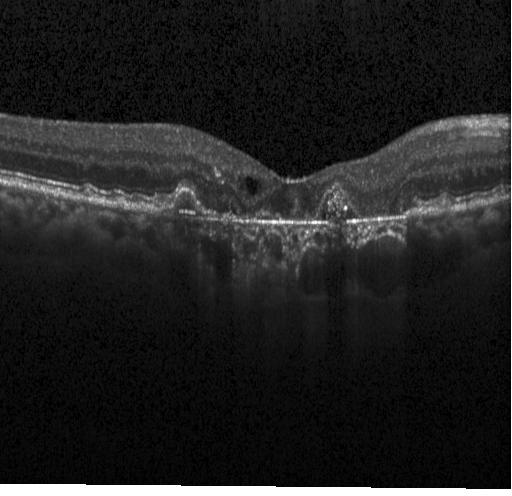
Through the macula · spectral-domain optical coherence tomography · Heidelberg Spectralis · retinal OCT B-scan.
Diagnosis: a choroidal neovascular membrane.